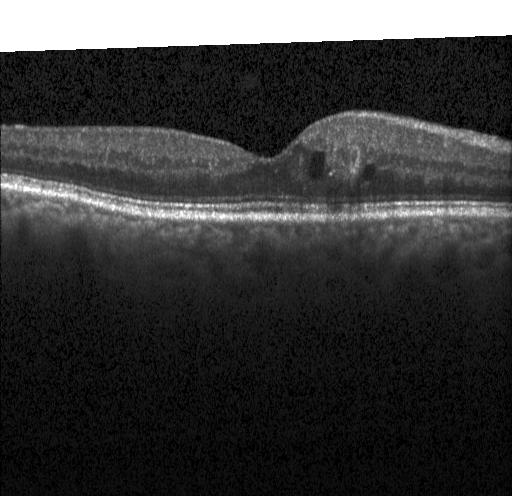 OCT B-scan · fovea-centered. Diagnosis: DME.